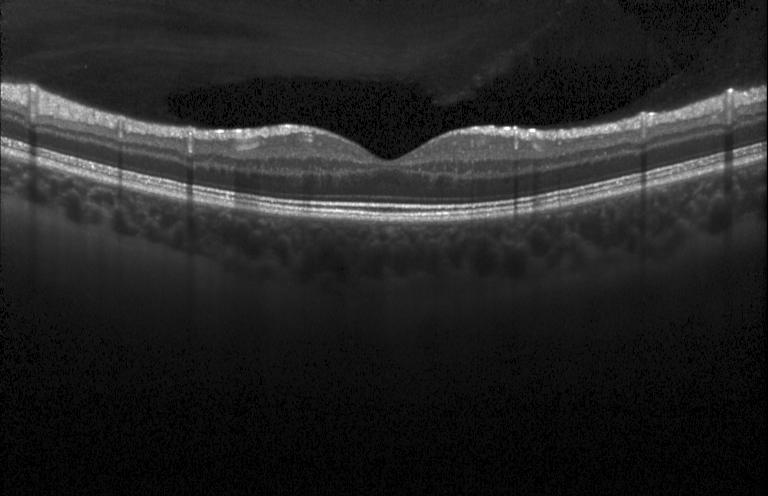
Impression: no choroidal neovascularization, diabetic macular edema, or drusen.